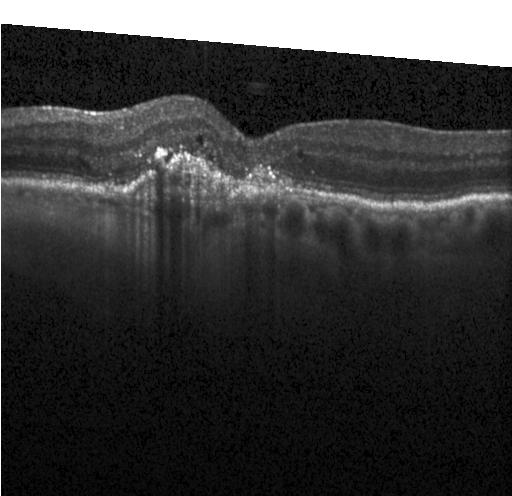

SD-OCT; fovea-centered; optical coherence tomography scan; instrument: Heidelberg Spectralis.
Finding: a choroidal neovascular membrane.